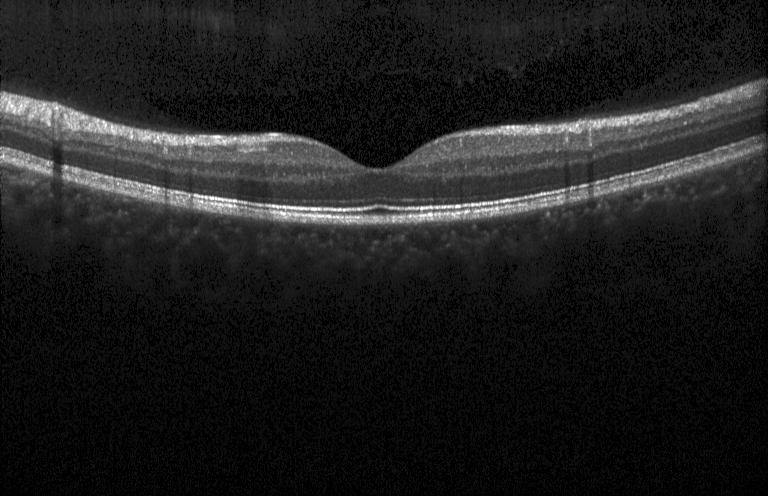
Spectral-domain OCT, through the macula, optical coherence tomography scan — Impression: no evidence of choroidal neovascularization, diabetic macular edema, or drusen.